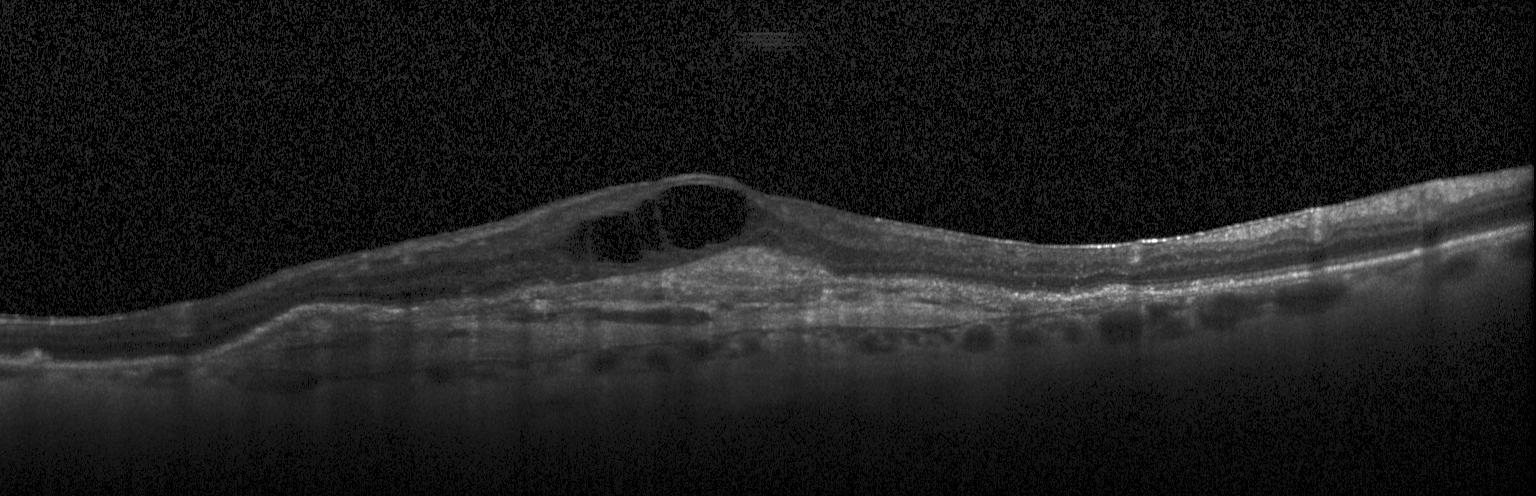
OCT scan showing CNV.